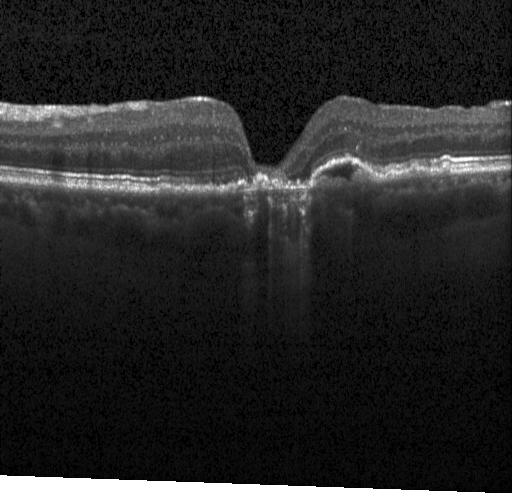 Optical coherence tomography scan · spectral-domain optical coherence tomography · centered on the fovea · acquired on a Heidelberg Spectralis
Finding: CNV.